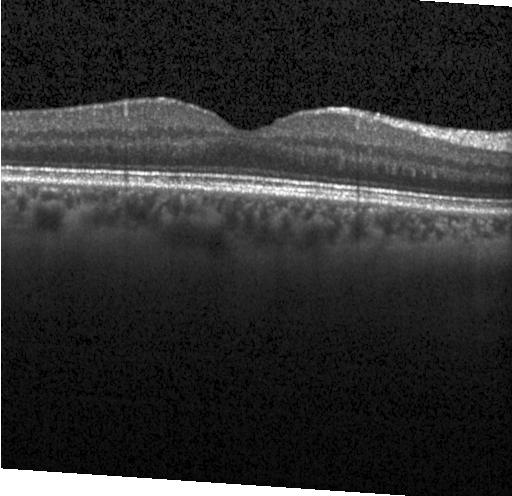

Optical coherence tomography scan · centered on the fovea. Diagnosis: no choroidal neovascularization, diabetic macular edema, or drusen.